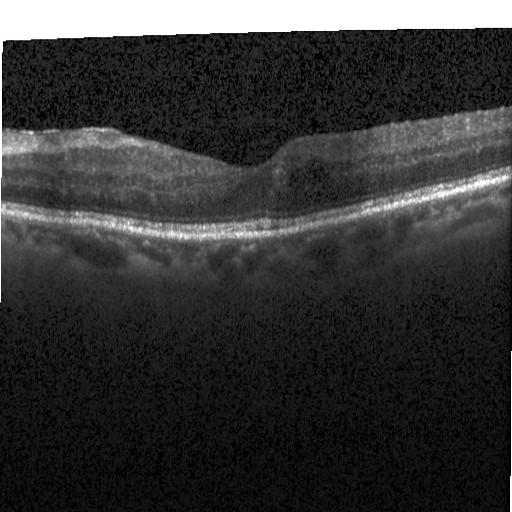 Assessment: DME.